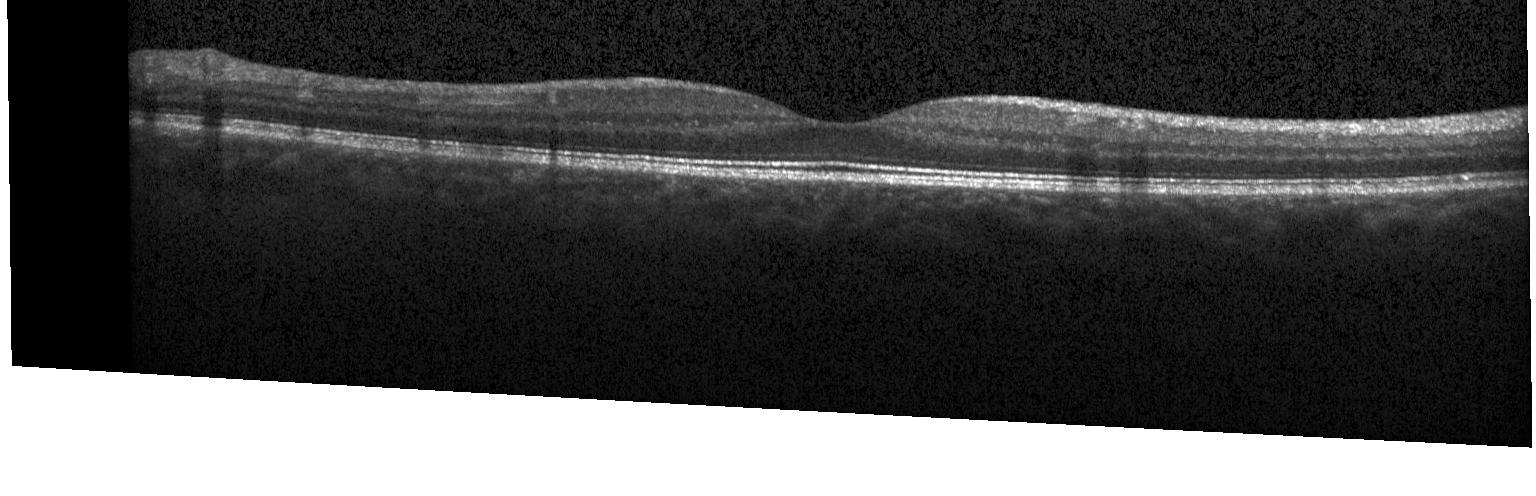
Optical coherence tomography B-scan.
Finding: no choroidal neovascularization, no diabetic macular edema, and no drusen.